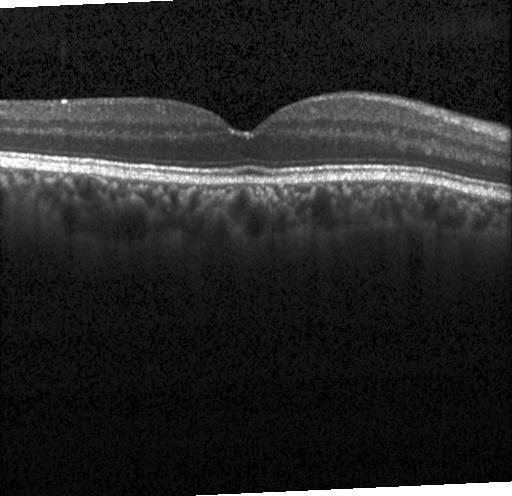

Optical coherence tomography scan; Heidelberg Spectralis OCT system — Diagnosis: no CNV, DME, or drusen.